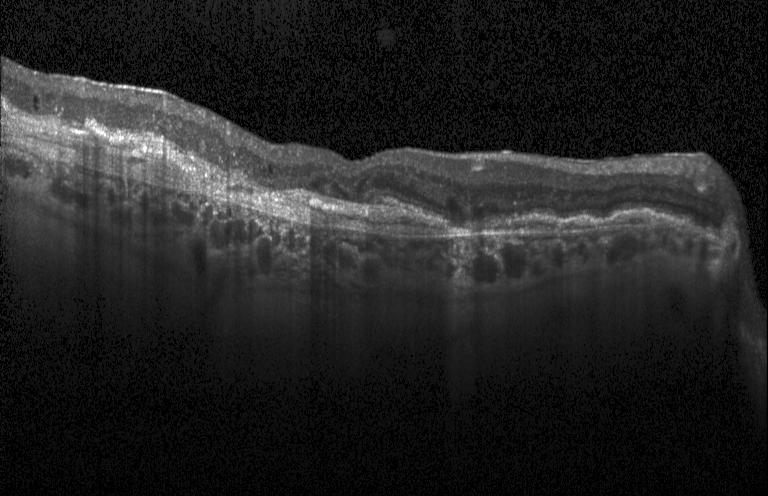
Finding: CNV.